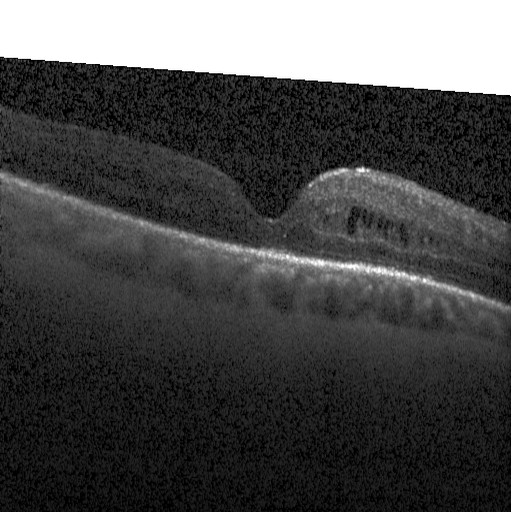

Optical coherence tomography scan. Centered on the fovea
OCT finding: diabetic macular edema (DME).